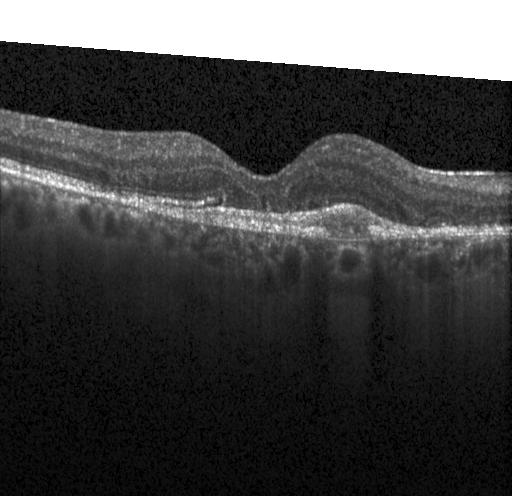

Spectral-domain optical coherence tomography · acquired on a Heidelberg Spectralis · centered on the fovea · OCT B-scan — Impression: a choroidal neovascular membrane.